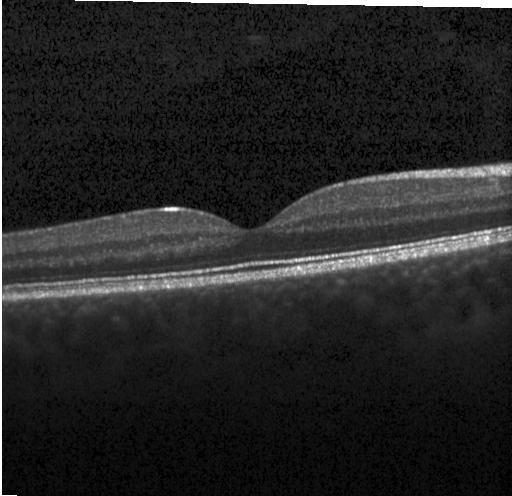

SD-OCT · retinal OCT B-scan
Impression: no choroidal neovascularization, no diabetic macular edema, and no drusen.